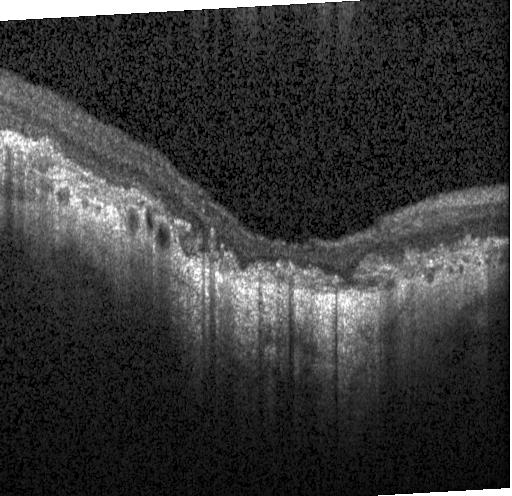

Acquired on a Heidelberg Spectralis, optical coherence tomography B-scan, spectral-domain optical coherence tomography — Macular OCT: choroidal neovascularization.